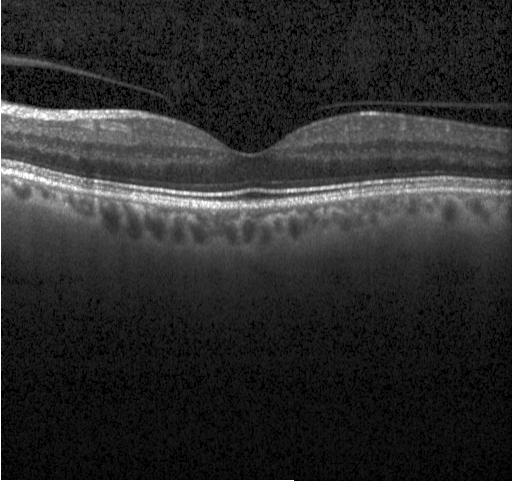
Retinal OCT cross-section. Dx: no choroidal neovascularization, no diabetic macular edema, and no drusen.